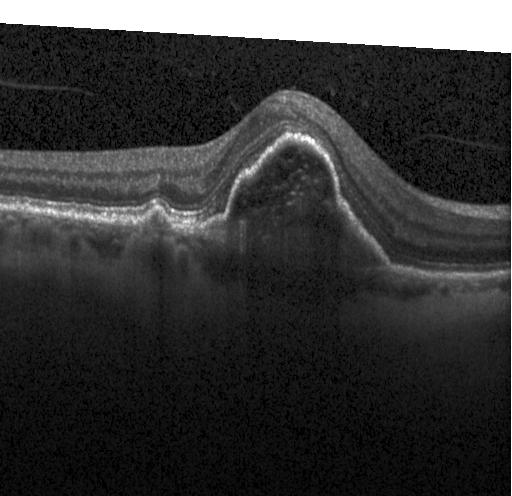
Optical coherence tomography scan. Instrument: Heidelberg Spectralis
Impression: a choroidal neovascular membrane.